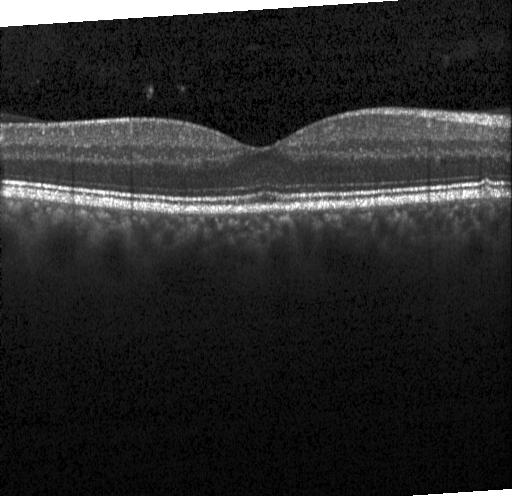 Optical coherence tomography scan, Heidelberg Spectralis OCT system. Finding: drusen.